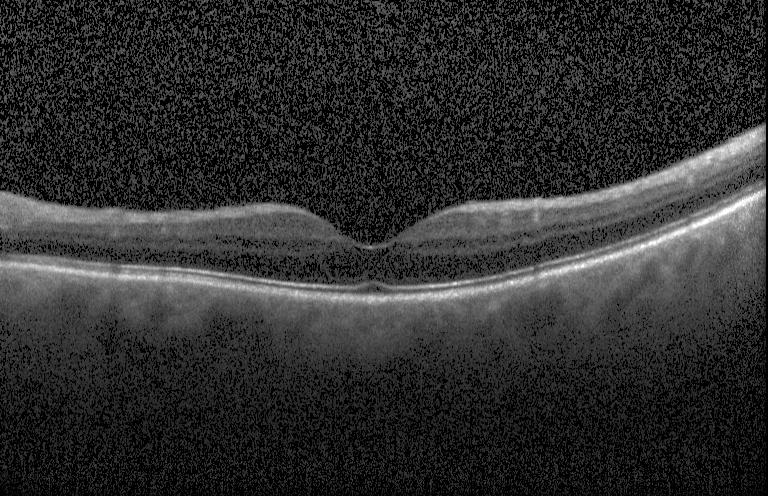 Impression: no choroidal neovascularization, diabetic macular edema, or drusen.